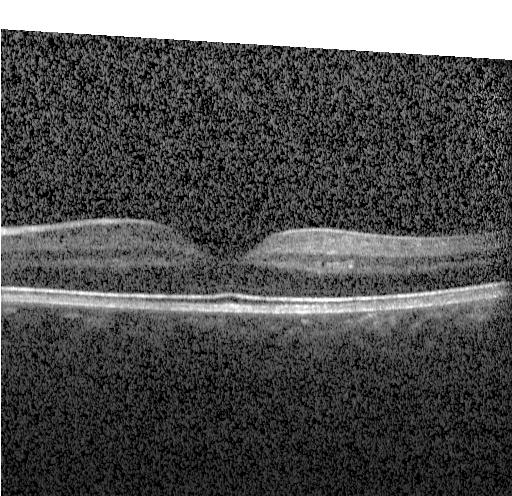 Macular OCT: no evidence of CNV, DME, or drusen.